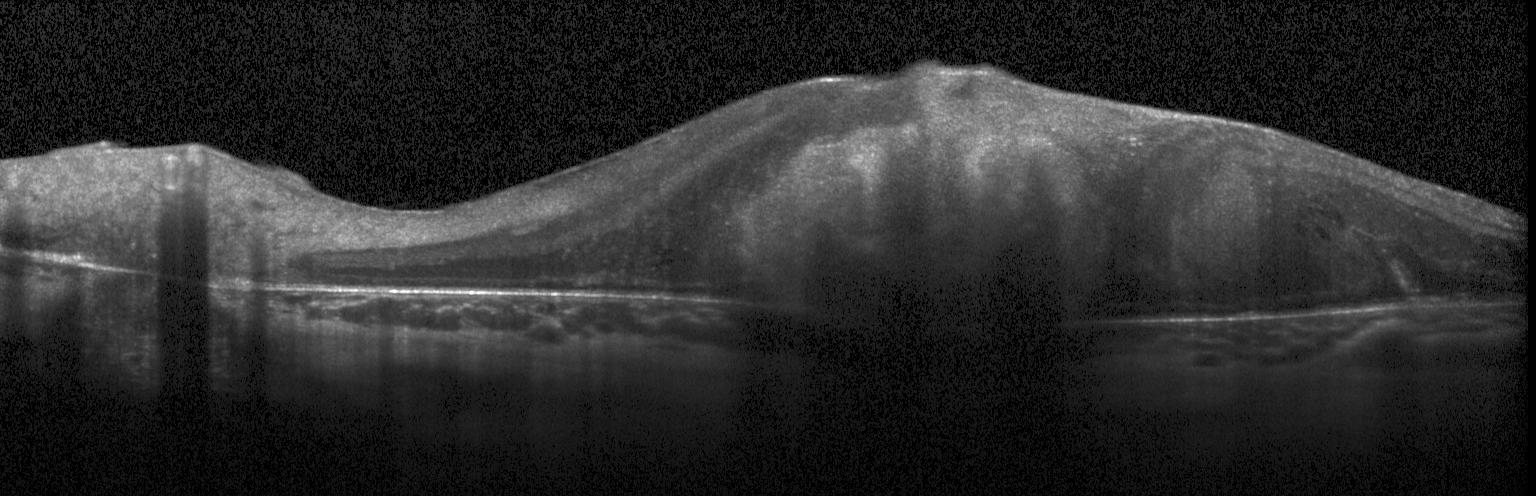 Dx: choroidal neovascularization (CNV).